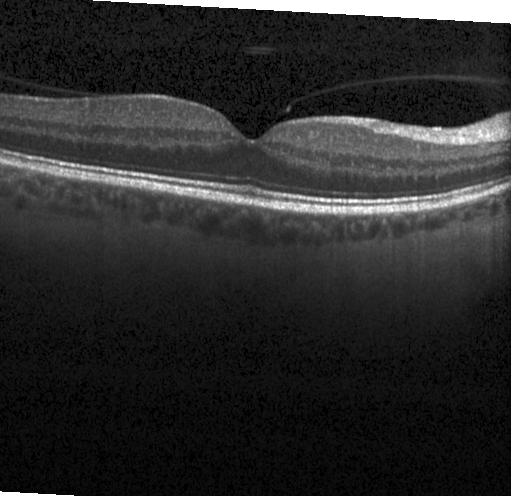
Acquired on a Heidelberg Spectralis · spectral-domain optical coherence tomography · centered on the fovea · retinal OCT cross-section. Macular OCT: no choroidal neovascularization, diabetic macular edema, or drusen.